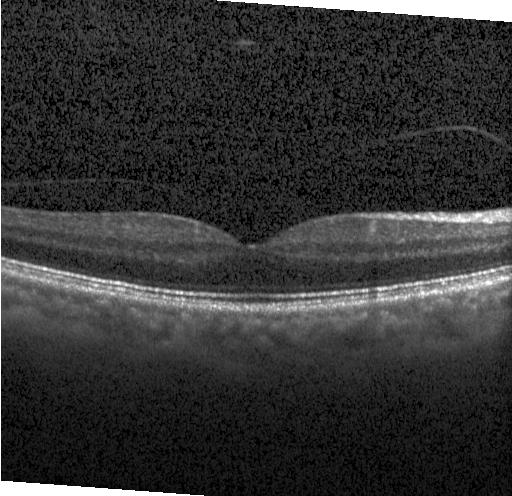
Retinal OCT cross-section. Instrument: Heidelberg Spectralis. Spectral-domain OCT.
Diagnosis: neither choroidal neovascularization, diabetic macular edema, nor drusen.